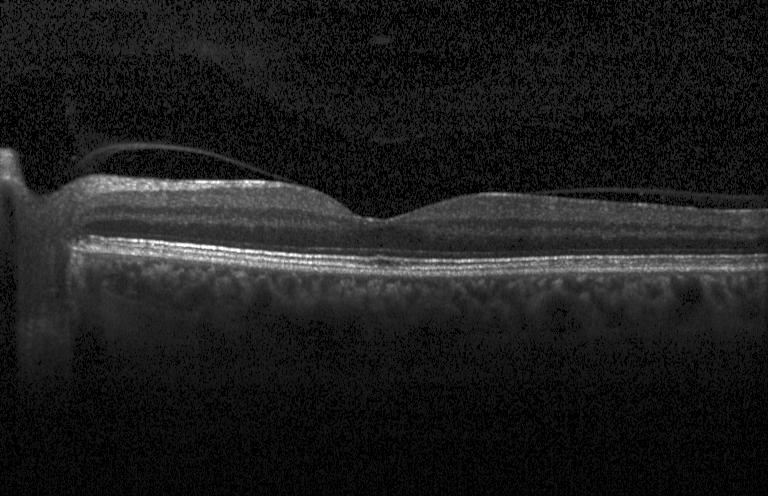

Macular OCT demonstrating neither choroidal neovascularization, diabetic macular edema, nor drusen.